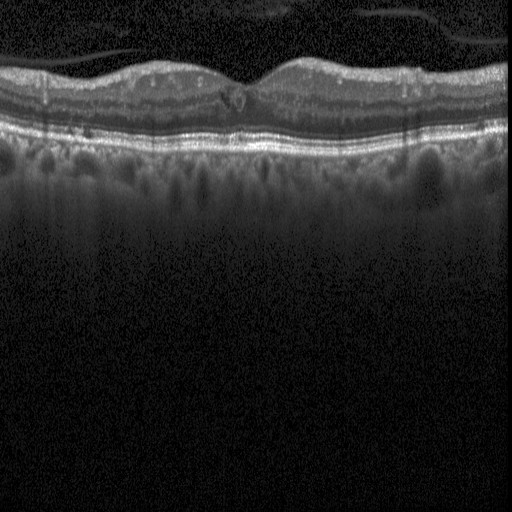
Dx: diabetic macular edema.